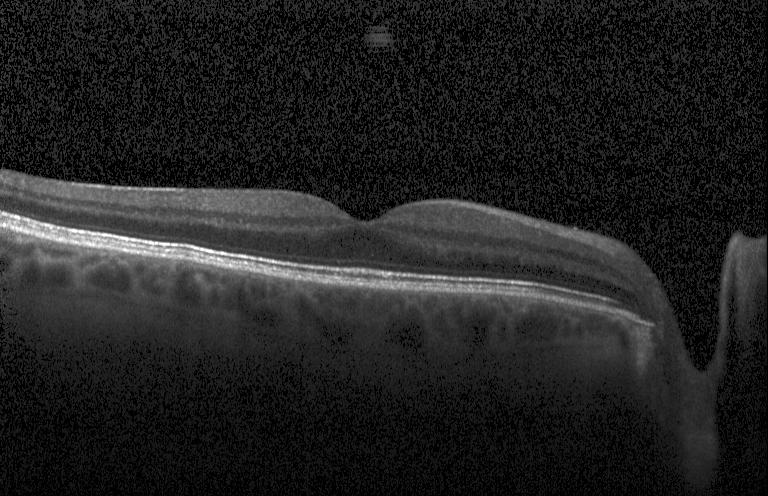

Fovea-centered, spectral-domain OCT, retinal OCT B-scan, acquired on a Heidelberg Spectralis
The scan shows neither choroidal neovascularization, diabetic macular edema, nor drusen.